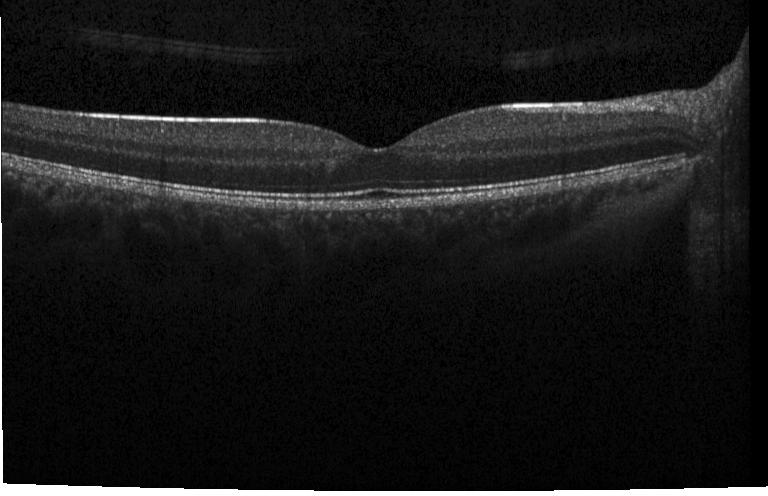 OCT finding: no choroidal neovascularization, diabetic macular edema, or drusen.